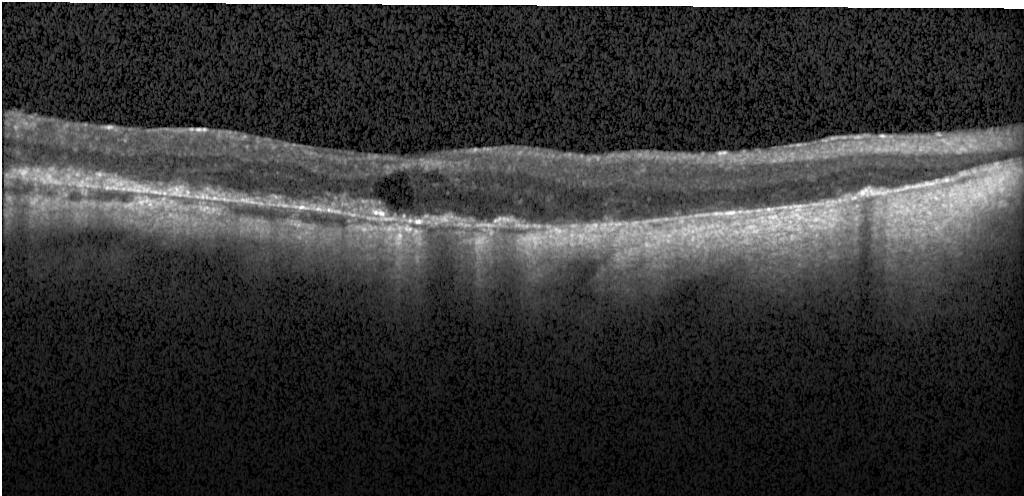
Retinal OCT cross-section
OCT finding: a choroidal neovascular membrane.